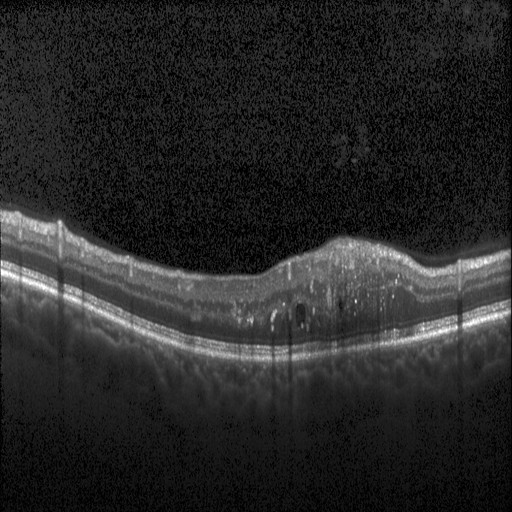 Heidelberg Spectralis OCT system, retinal OCT B-scan — The scan shows diabetic macular edema.